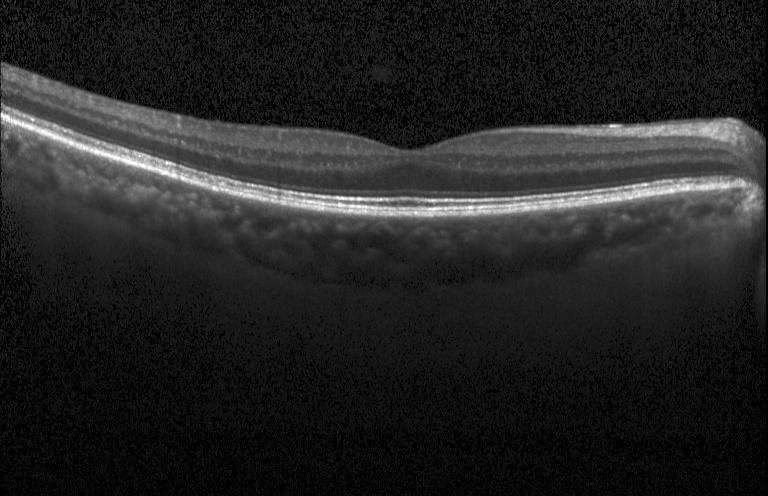

Spectral-domain optical coherence tomography · horizontal scan through the fovea · optical coherence tomography scan · Heidelberg Spectralis — OCT finding: no choroidal neovascularization, no diabetic macular edema, and no drusen.